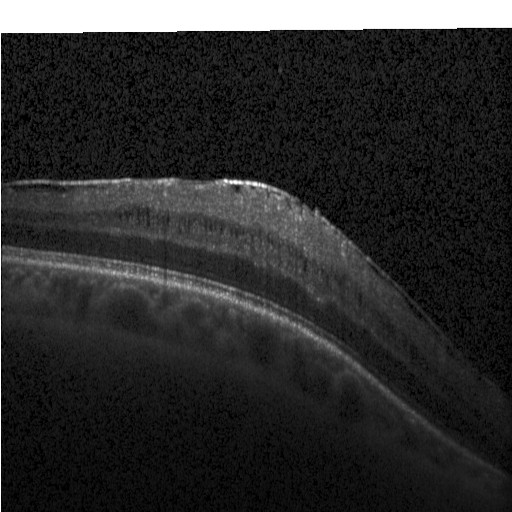

This B-scan demonstrates diabetic macular edema.